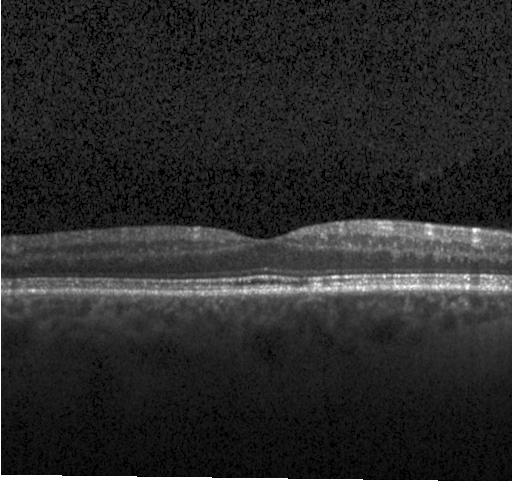

OCT line scan · centered on the fovea · spectral-domain OCT
Diagnosis: no CNV, no DME, and no drusen.